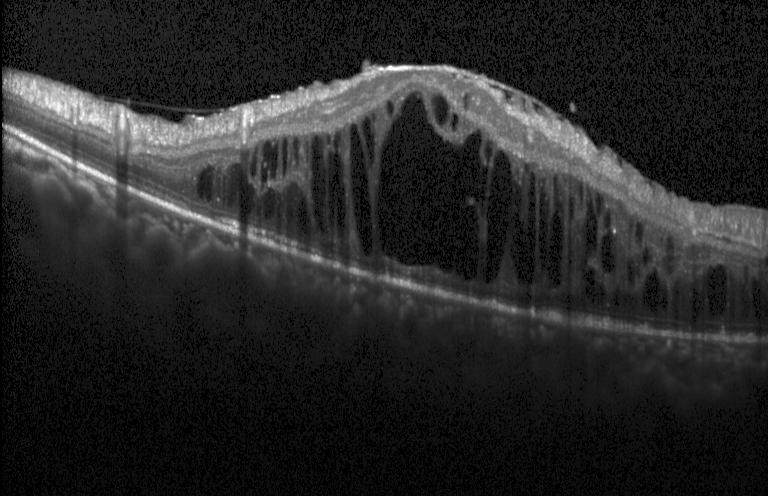

Retinal OCT cross-section. Heidelberg Spectralis OCT system. Spectral-domain OCT
The scan shows diabetic macular edema (DME).